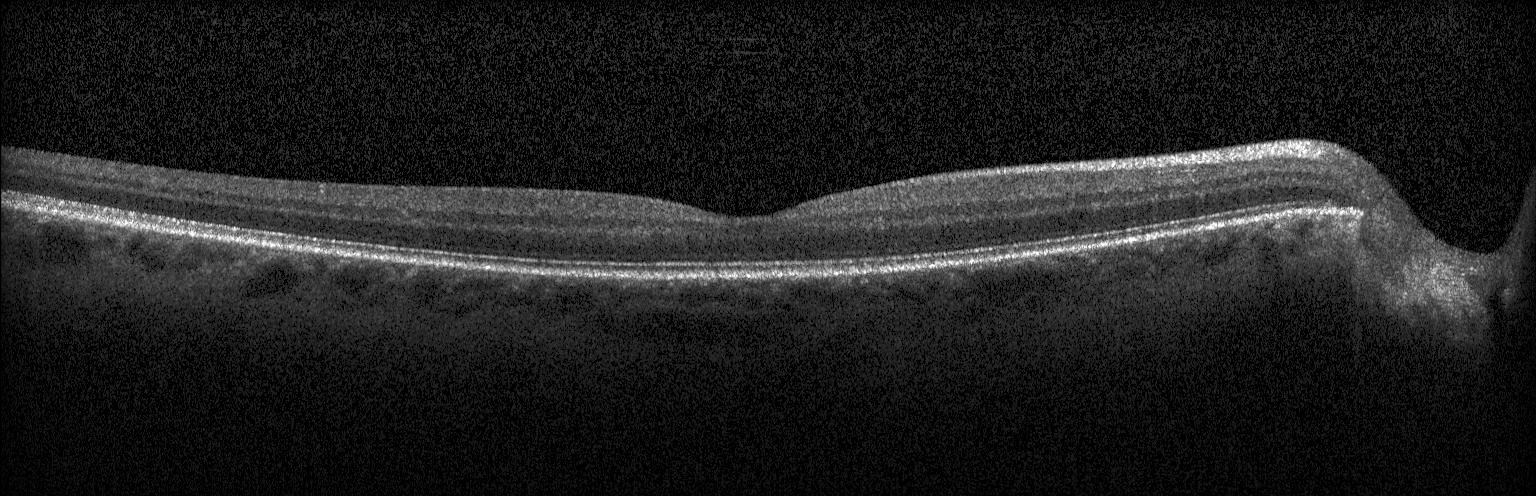 The scan shows no choroidal neovascularization, no diabetic macular edema, and no drusen.